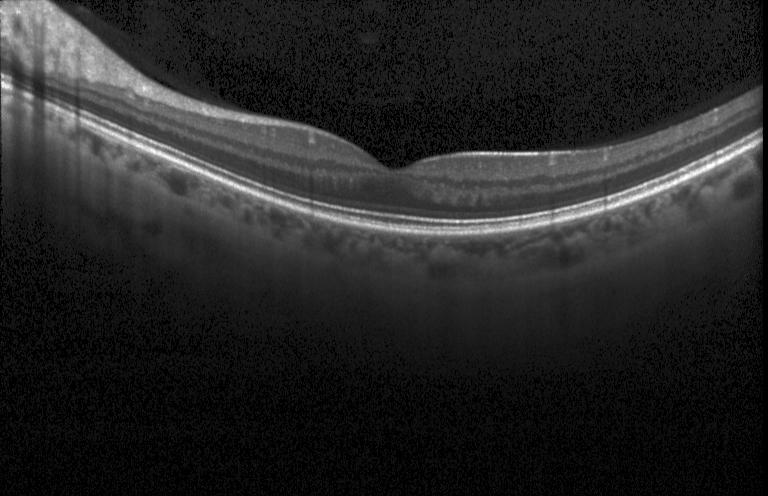

Impression: neither CNV, DME, nor drusen.